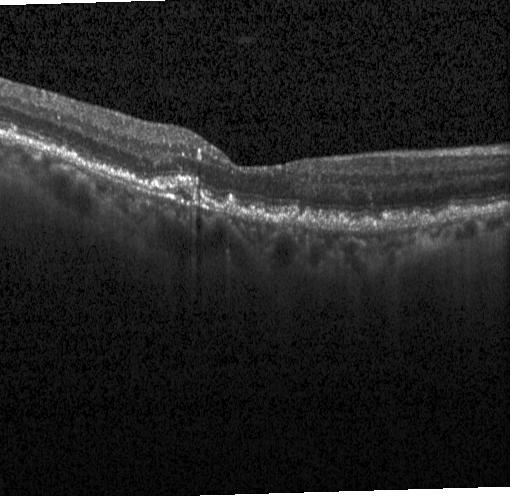 Optical coherence tomography scan.
Impression: a choroidal neovascular membrane.